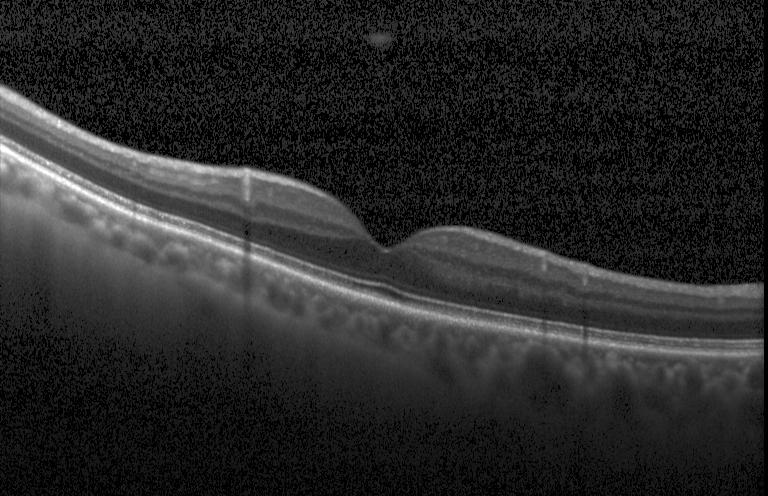
Finding: no CNV, no DME, and no drusen.